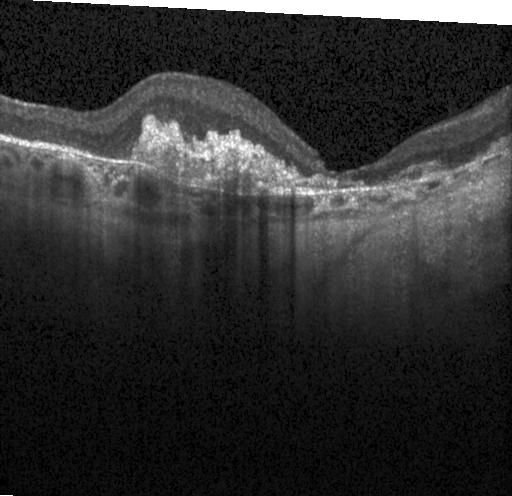
Horizontal scan through the fovea. OCT line scan. Spectral-domain optical coherence tomography — Dx: a choroidal neovascular membrane.